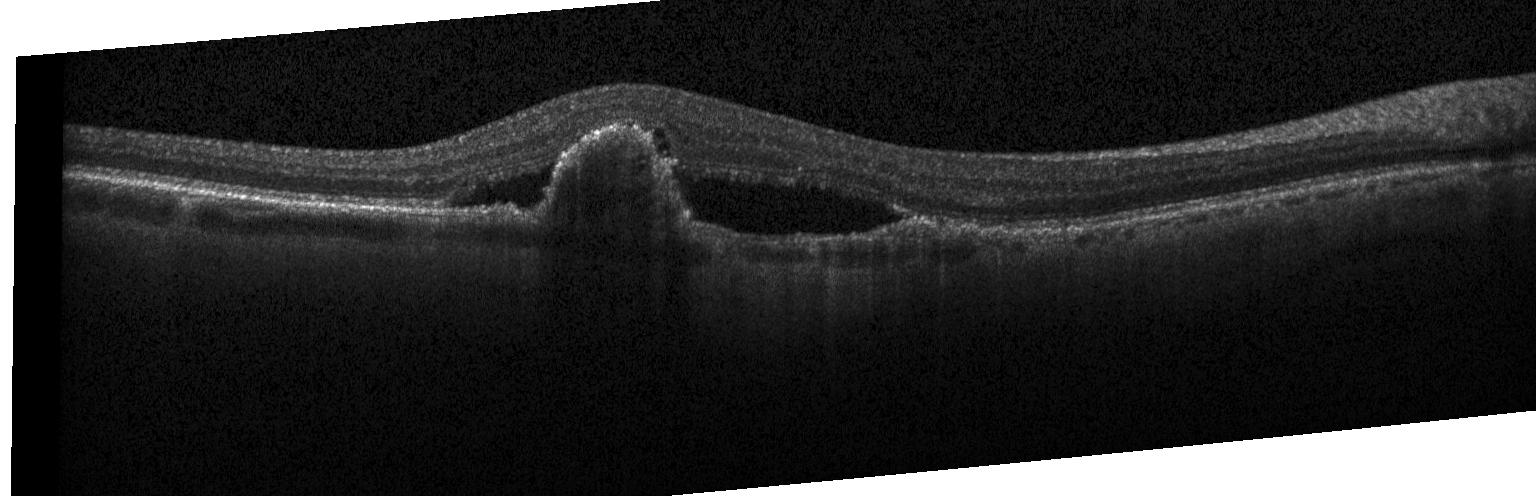
Impression: a choroidal neovascular membrane.